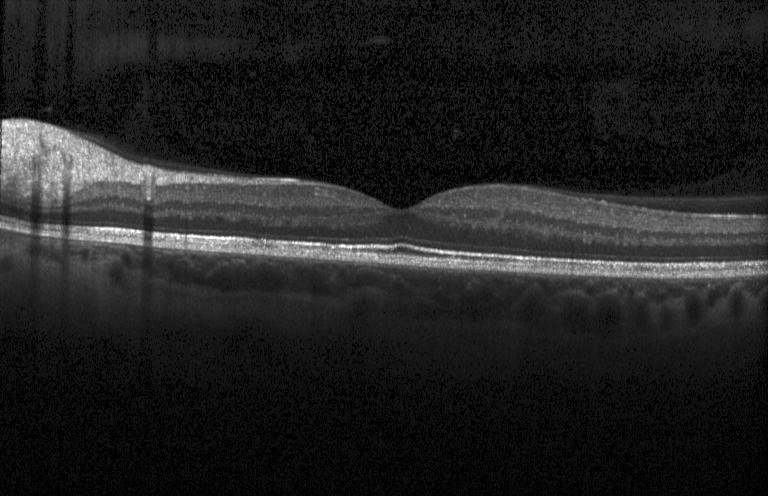

Retinal OCT B-scan
Diagnosis: no choroidal neovascularization, diabetic macular edema, or drusen.